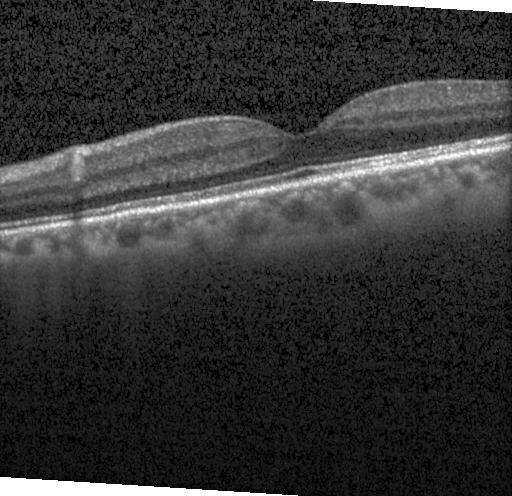

OCT line scan.
No CNV, no DME, and no drusen.